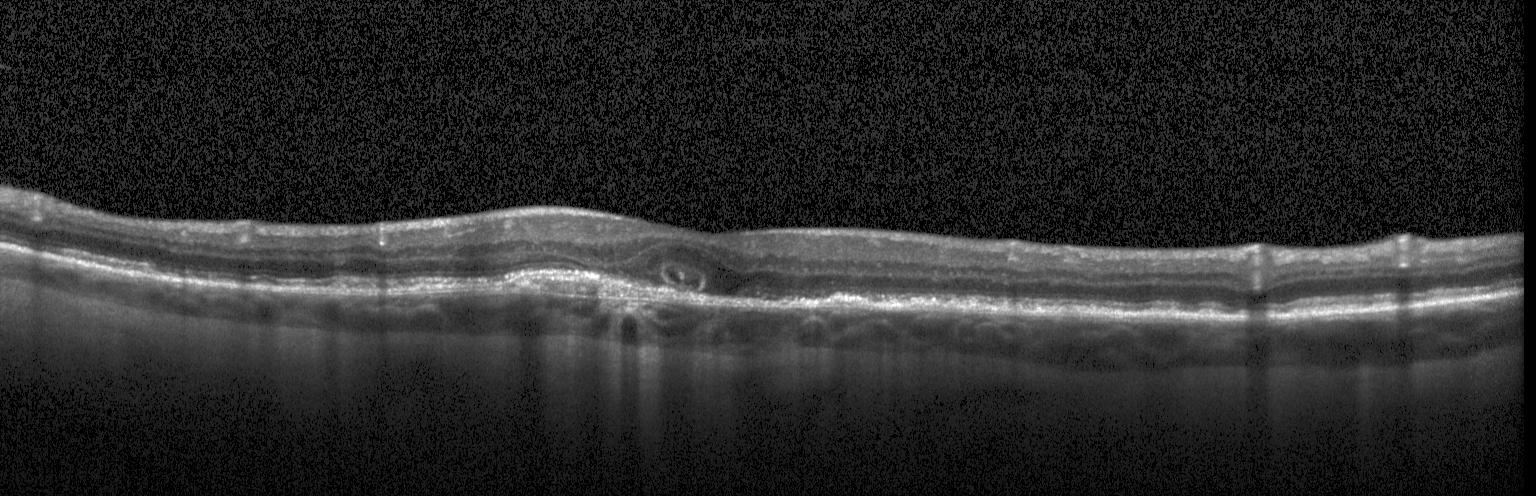
Retinal OCT cross-section showing choroidal neovascularization (CNV).